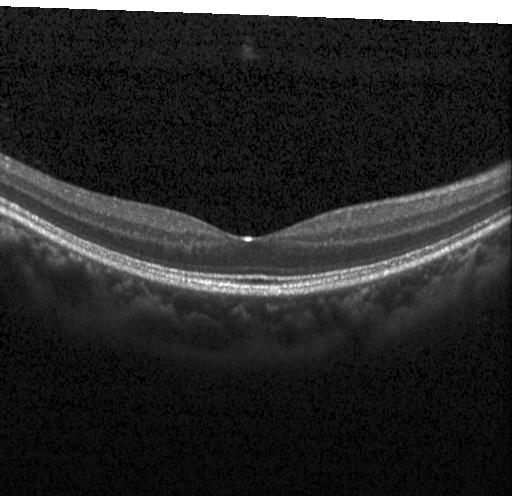
Retinal OCT B-scan; horizontal scan through the fovea.
Diagnosis: no evidence of choroidal neovascularization, diabetic macular edema, or drusen.